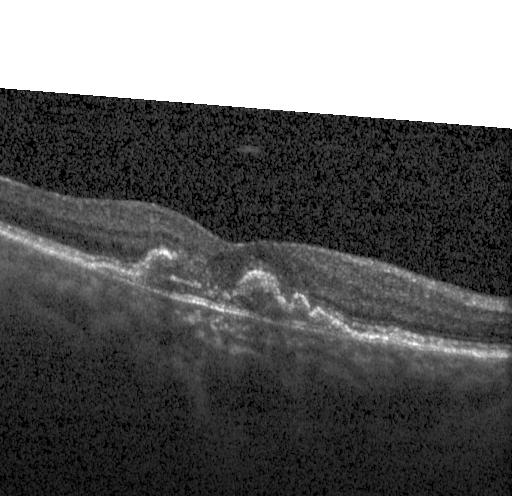
Retinal OCT cross-section showing choroidal neovascularization (CNV).